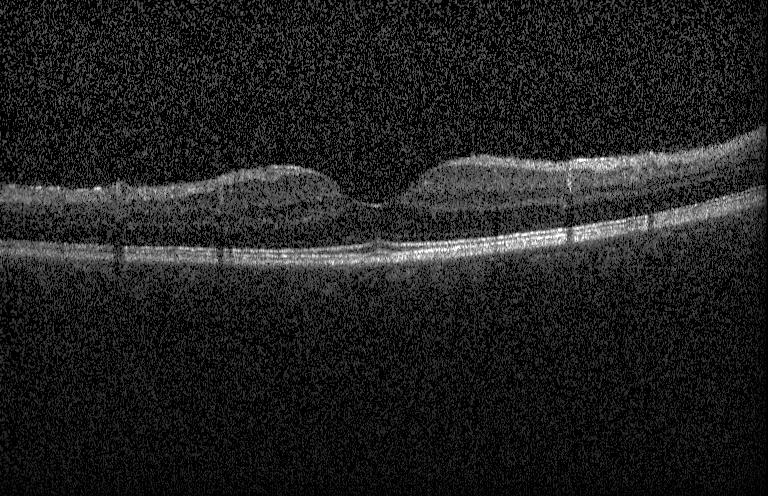 Heidelberg Spectralis, OCT B-scan
Diagnosis: neither choroidal neovascularization, diabetic macular edema, nor drusen.